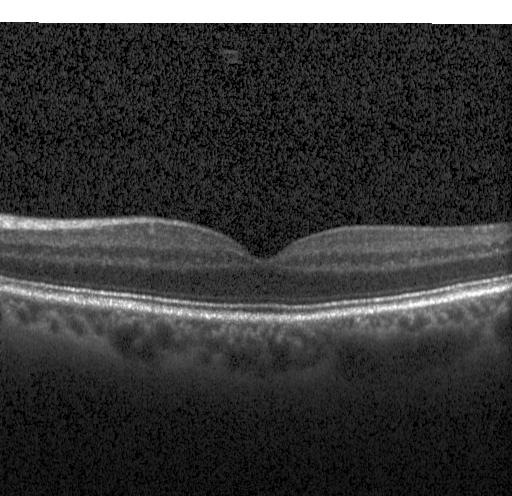 Retinal OCT B-scan. OCT finding: no evidence of choroidal neovascularization, diabetic macular edema, or drusen.